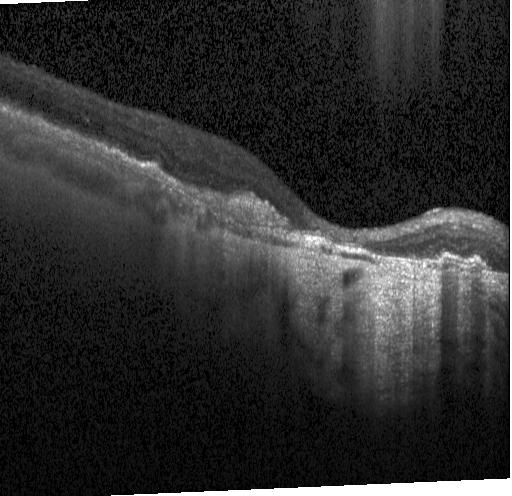
Macular OCT demonstrating a choroidal neovascular membrane.